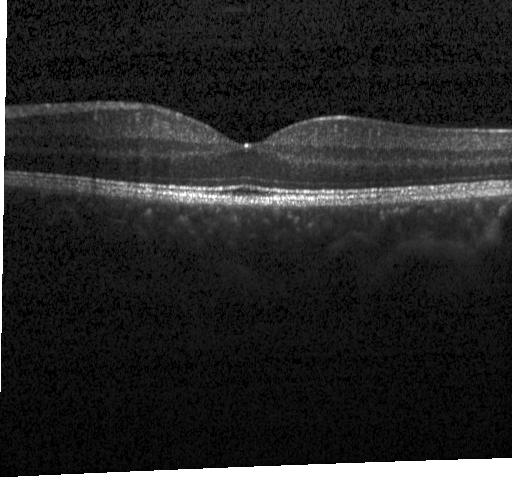 No evidence of CNV, DME, or drusen.